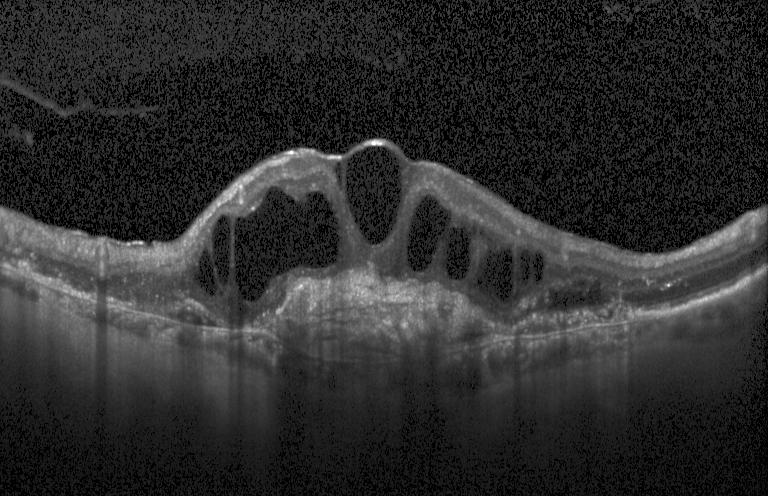 Retinal OCT cross-section.
Impression: a choroidal neovascular membrane.